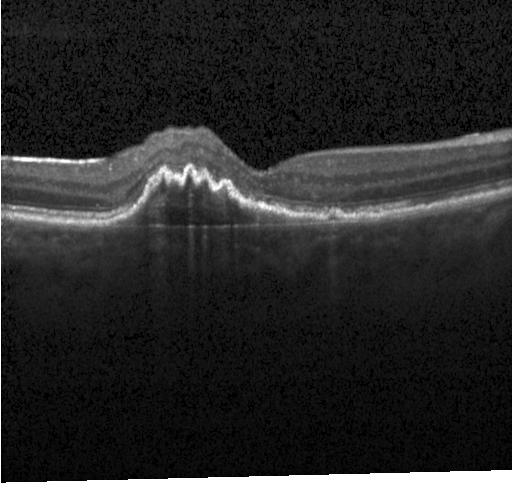
OCT line scan.
Impression: a choroidal neovascular membrane.